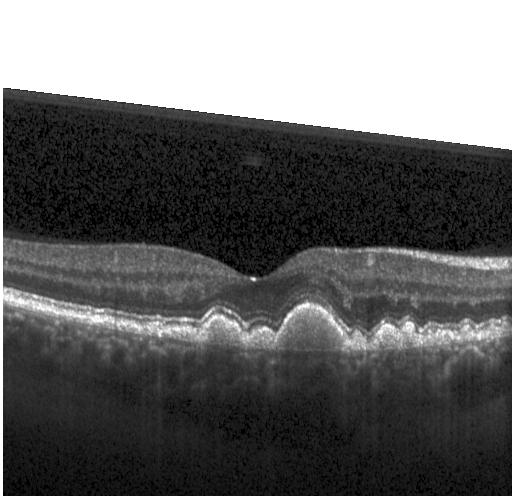 SD-OCT; OCT B-scan; instrument: Heidelberg Spectralis. Diagnosis: multiple drusen.